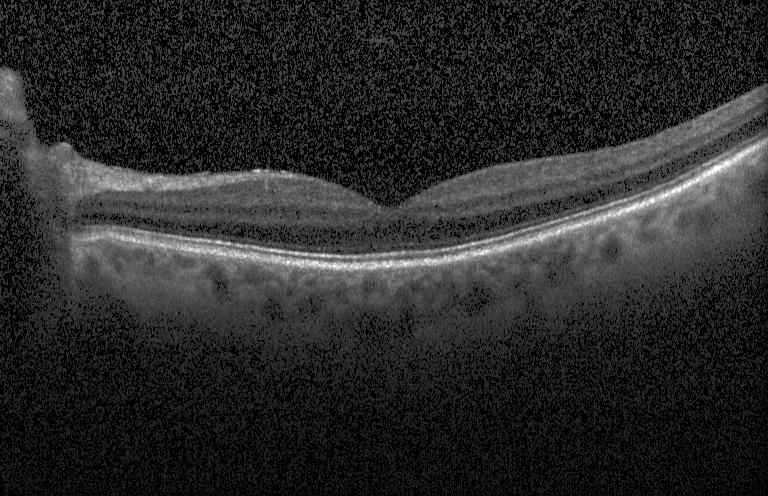
Retinal OCT B-scan. SD-OCT.
Macular OCT: no CNV, no DME, and no drusen.